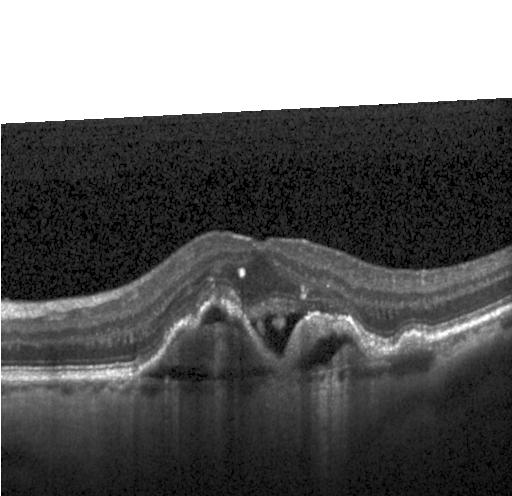 Dx: a choroidal neovascular membrane.